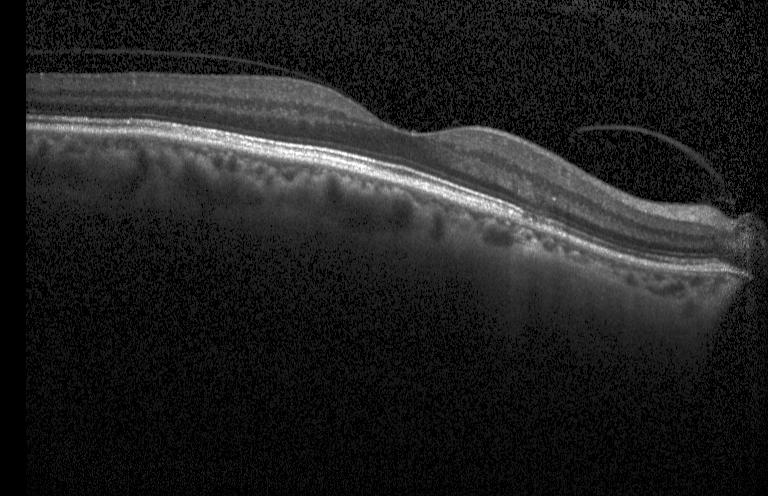 Spectral-domain optical coherence tomography. Macular scan. OCT line scan
Macular OCT: no choroidal neovascularization, no diabetic macular edema, and no drusen.